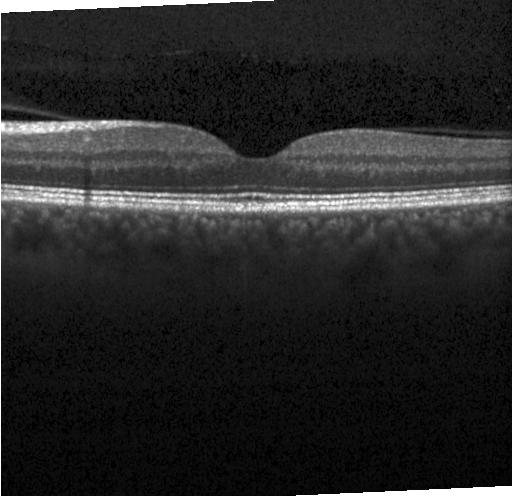 Spectral-domain OCT · optical coherence tomography B-scan · through the macula · Heidelberg Spectralis
OCT finding: no CNV, no DME, and no drusen.